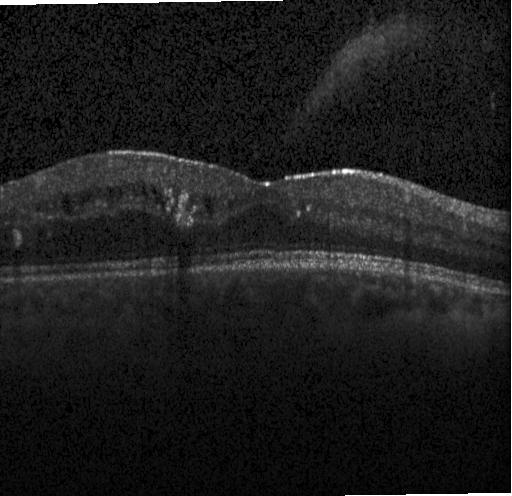 SD-OCT; centered on the fovea; retinal OCT cross-section; Heidelberg Spectralis. Finding: DME.